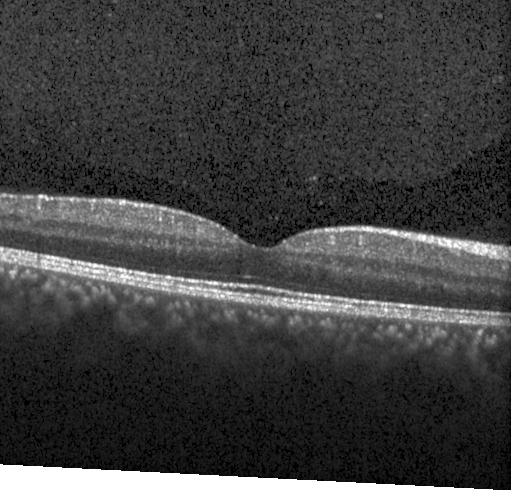
OCT B-scan. Diagnosis: no evidence of CNV, DME, or drusen.